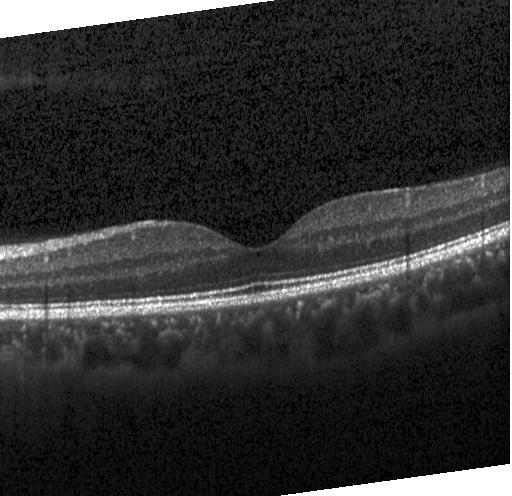

OCT line scan. Impression: neither choroidal neovascularization, diabetic macular edema, nor drusen.